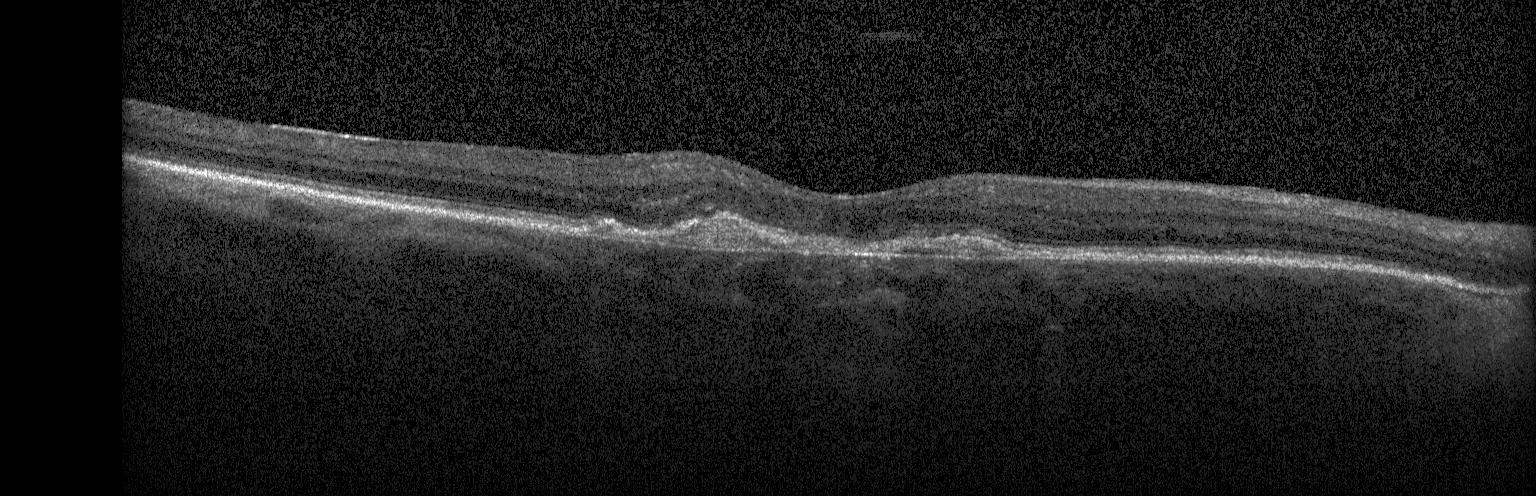
OCT B-scan showing a choroidal neovascular membrane.